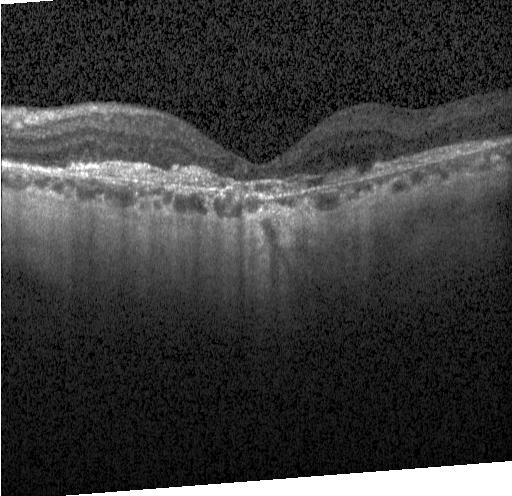
Centered on the fovea. Optical coherence tomography B-scan.
Macular OCT: CNV.